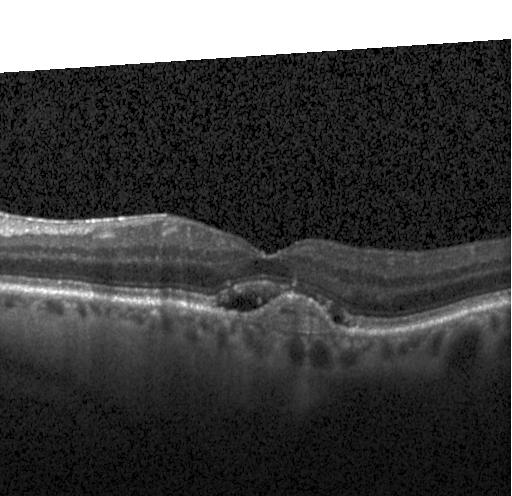

Instrument: Heidelberg Spectralis; OCT B-scan; fovea-centered; spectral-domain optical coherence tomography.
Finding: choroidal neovascularization (CNV).